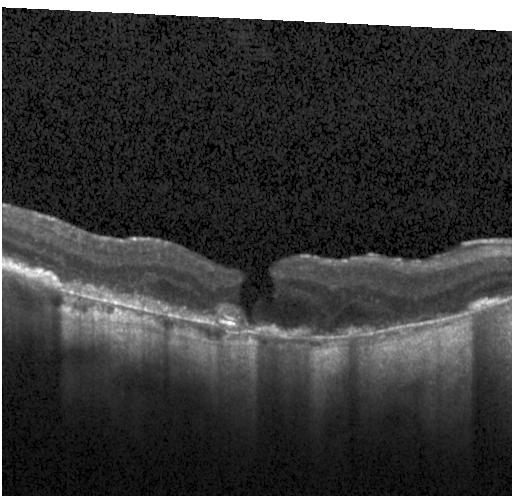 OCT B-scan showing choroidal neovascularization (CNV).